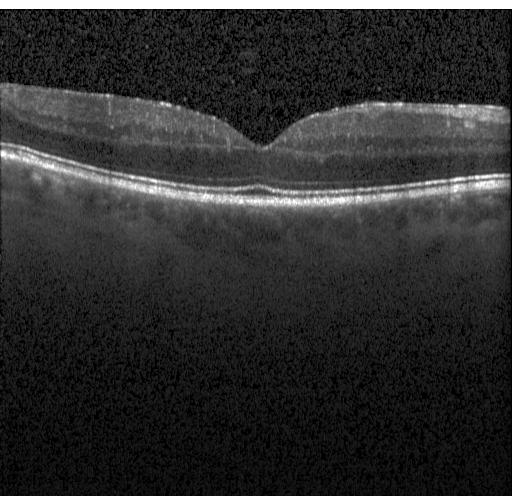

Impression: neither CNV, DME, nor drusen.